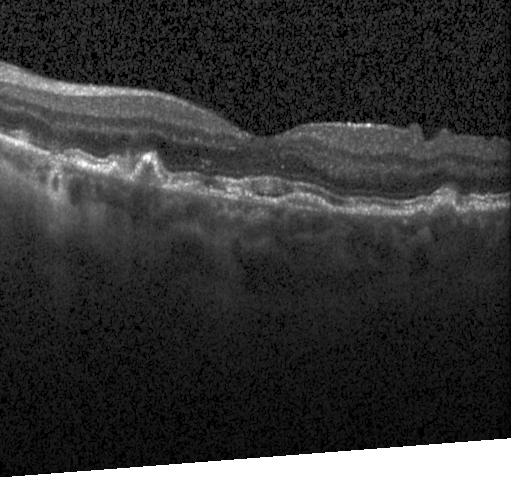

Retinal OCT cross-section. Impression: choroidal neovascularization.